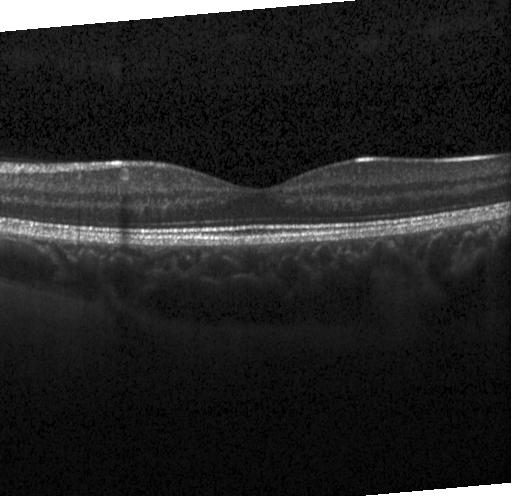 Optical coherence tomography scan, Heidelberg Spectralis OCT system, fovea-centered, SD-OCT
No evidence of choroidal neovascularization, diabetic macular edema, or drusen.